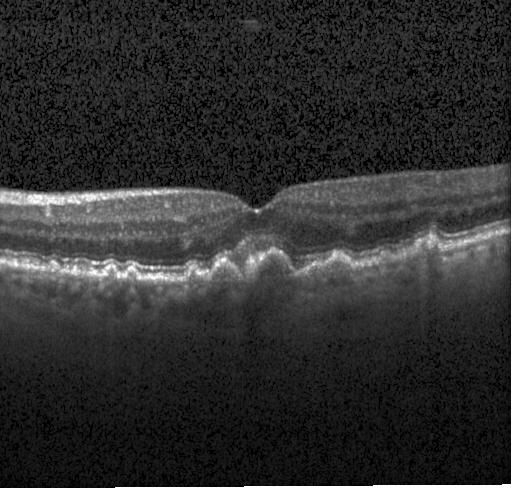
Macular OCT demonstrating multiple drusen.